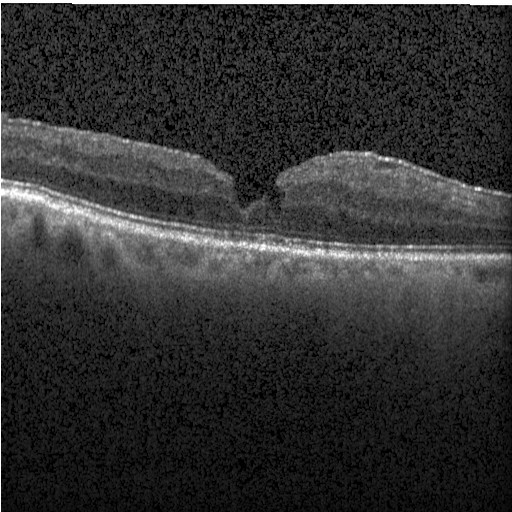

OCT line scan
Finding: diabetic macular edema.